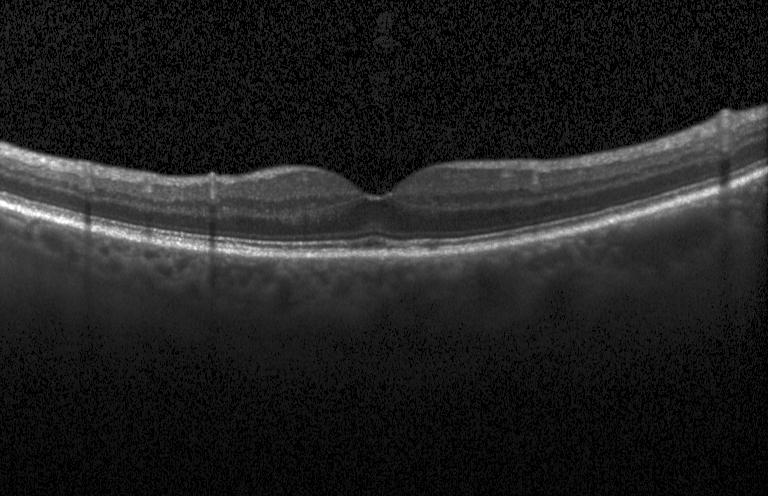
Through the macula; Heidelberg Spectralis OCT system; OCT line scan; spectral-domain optical coherence tomography — The scan shows neither choroidal neovascularization, diabetic macular edema, nor drusen.